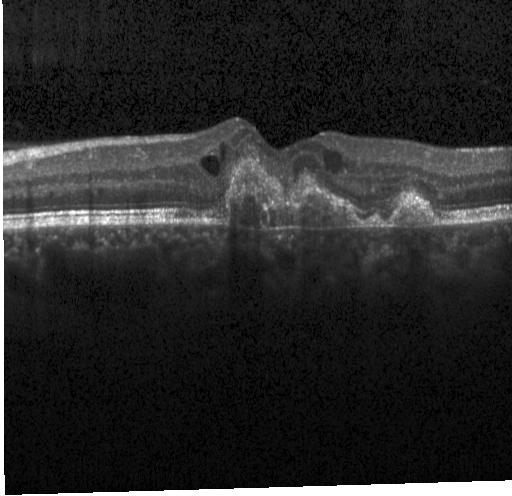
Retinal OCT cross-section
Assessment: a choroidal neovascular membrane.